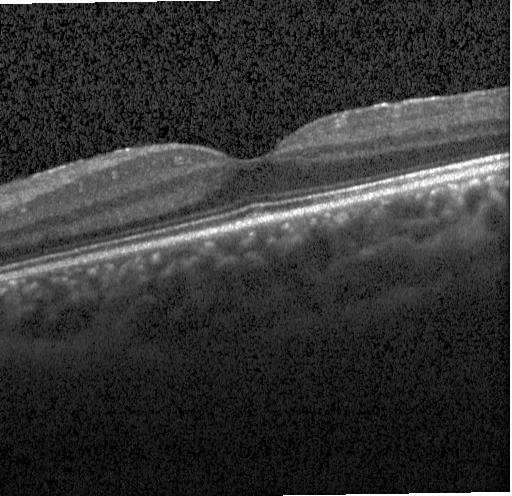
OCT B-scan.
Macular OCT: neither CNV, DME, nor drusen.